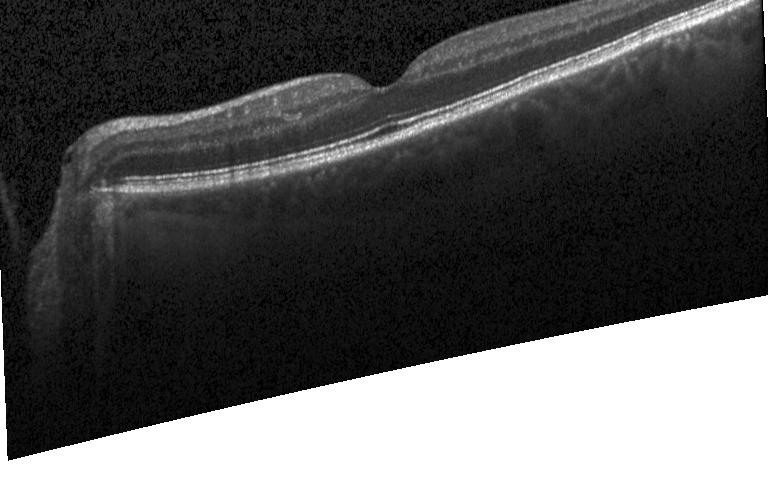
Horizontal scan through the fovea, retinal OCT B-scan, instrument: Heidelberg Spectralis, spectral-domain OCT — Impression: no evidence of choroidal neovascularization, diabetic macular edema, or drusen.